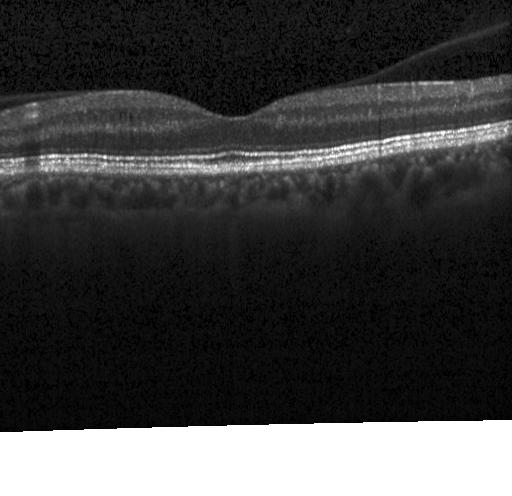

Retinal OCT cross-section
Diagnosis: no evidence of CNV, DME, or drusen.